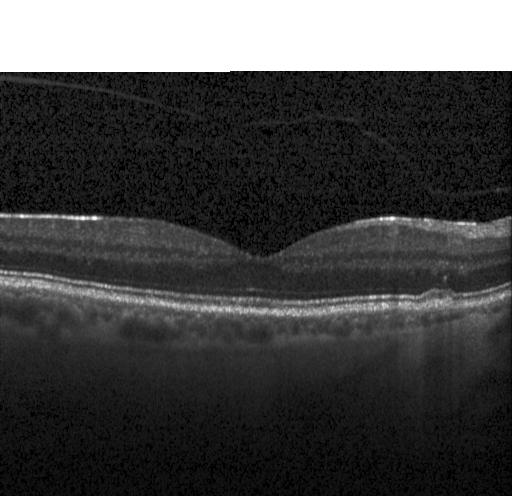
Centered on the fovea; optical coherence tomography scan.
Dx: drusen.